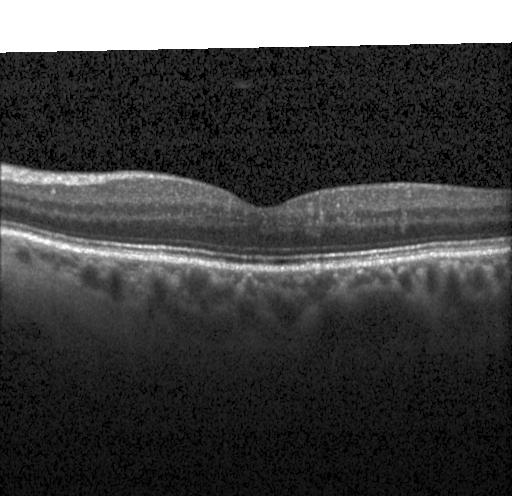
OCT line scan — Impression: neither CNV, DME, nor drusen.